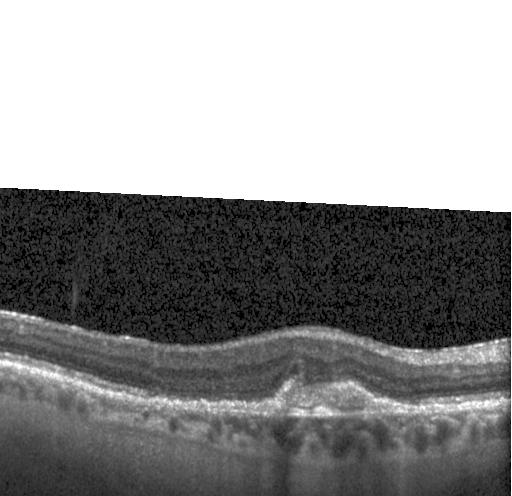

Optical coherence tomography scan. Heidelberg Spectralis OCT system. Spectral-domain OCT. Macular scan — Impression: a choroidal neovascular membrane.